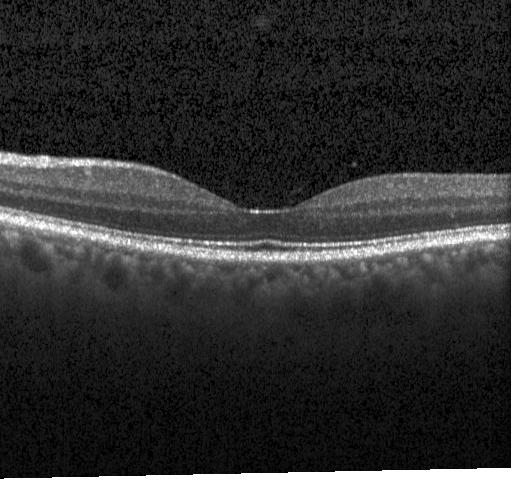 OCT B-scan. OCT finding: no choroidal neovascularization, diabetic macular edema, or drusen.